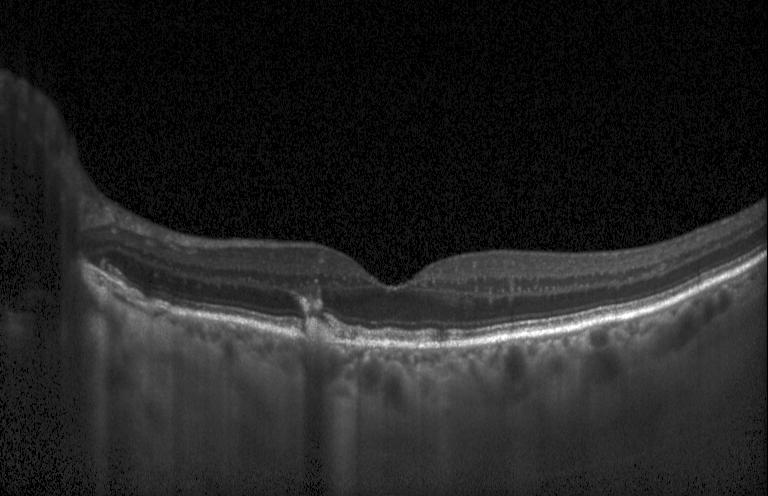

Heidelberg Spectralis OCT system; SD-OCT; retinal OCT B-scan
Diagnosis: multiple drusen.